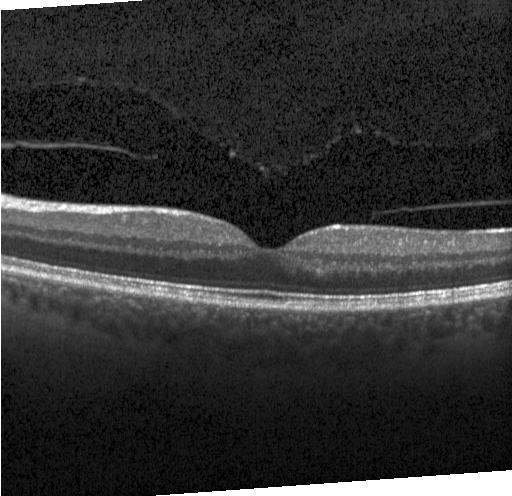

Heidelberg Spectralis, OCT B-scan, spectral-domain OCT, through the macula — Diagnosis: no CNV, no DME, and no drusen.